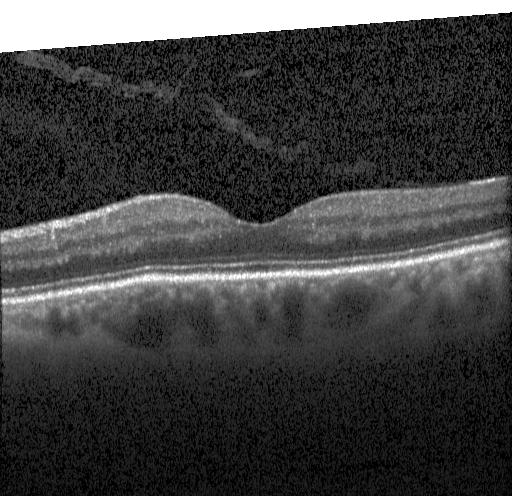 Retinal OCT cross-section
Finding: no choroidal neovascularization, diabetic macular edema, or drusen.